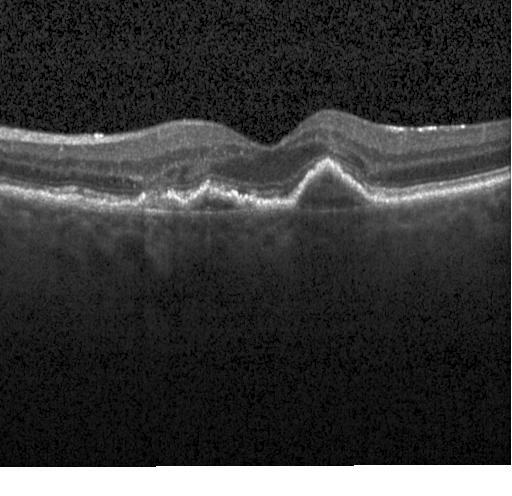
Diagnosis: a choroidal neovascular membrane.